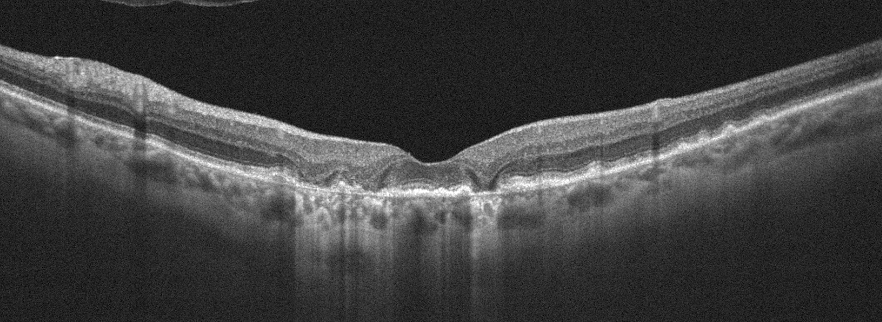
Instrument: Optovue Avanti RTVue XR; OCT B-scan; fovea-centered — The scan shows age-related macular degeneration (AMD).